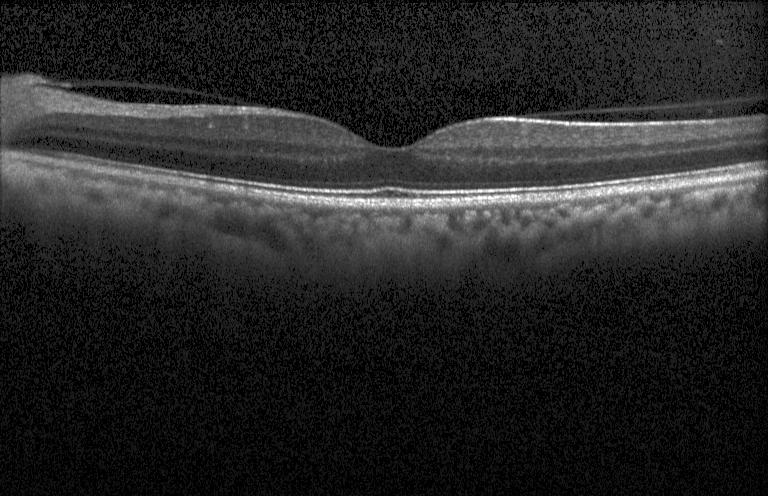

Diagnosis: no choroidal neovascularization, diabetic macular edema, or drusen.